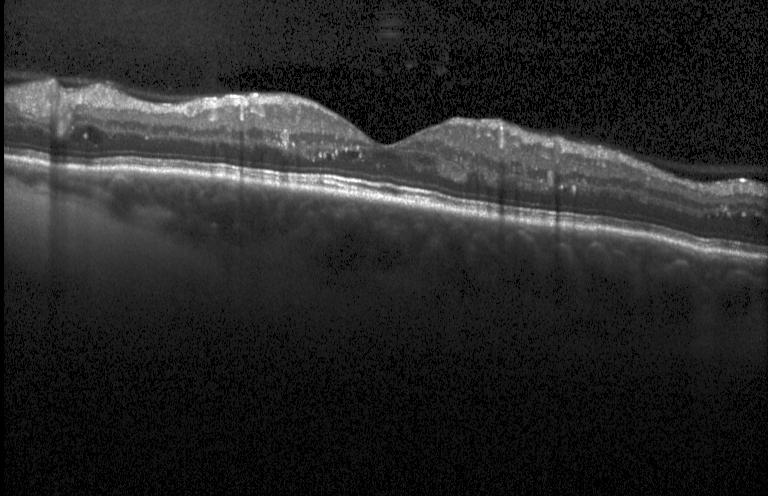
Centered on the fovea, Heidelberg Spectralis OCT system, retinal OCT B-scan, spectral-domain OCT
DME.